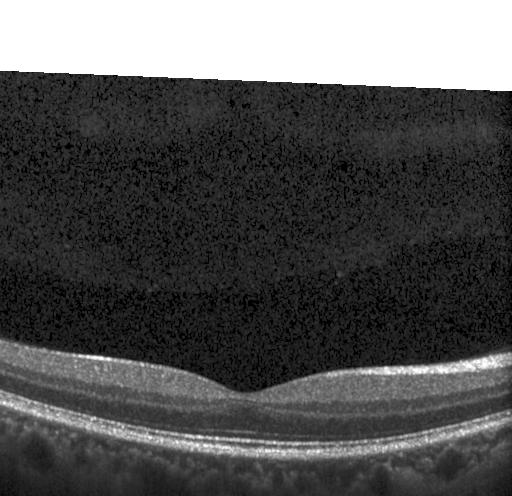
Through the macula; spectral-domain optical coherence tomography; instrument: Heidelberg Spectralis; OCT line scan
Finding: neither choroidal neovascularization, diabetic macular edema, nor drusen.